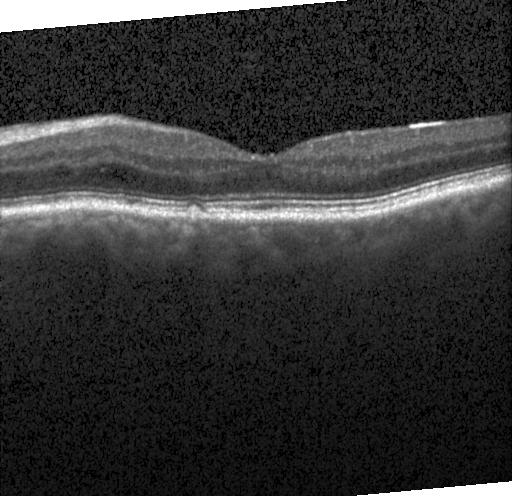
Retinal OCT cross-section, fovea-centered, spectral-domain optical coherence tomography
Finding: drusen.